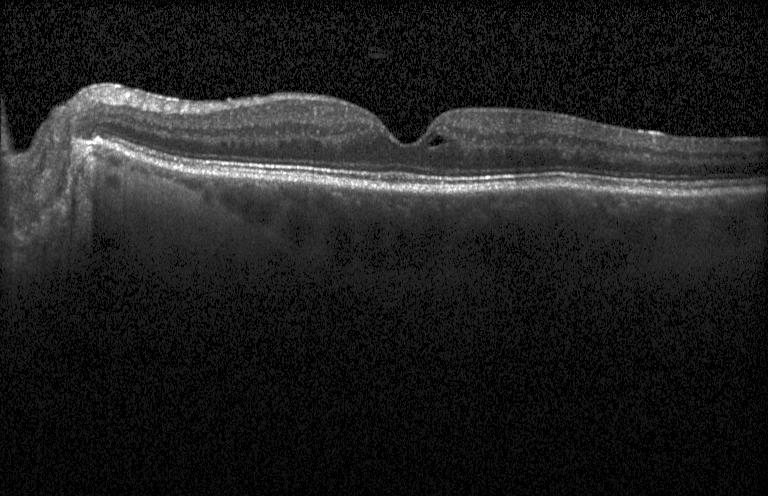
Heidelberg Spectralis · spectral-domain OCT · retinal OCT B-scan
This B-scan demonstrates diabetic macular edema (DME).